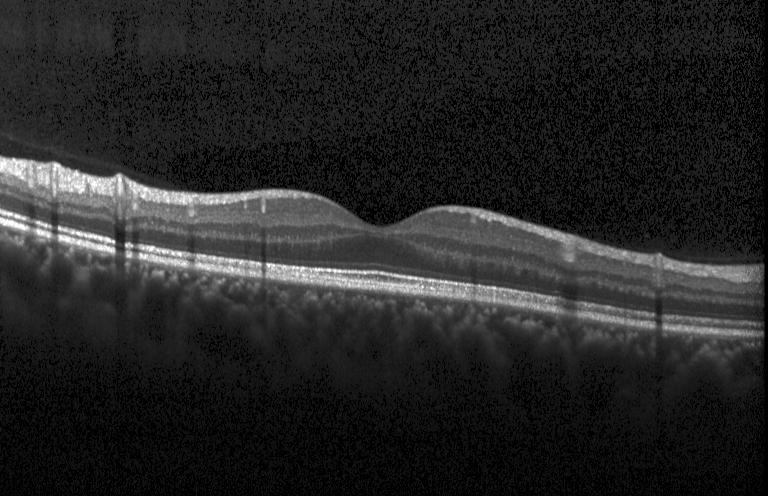
OCT line scan
Impression: neither CNV, DME, nor drusen.